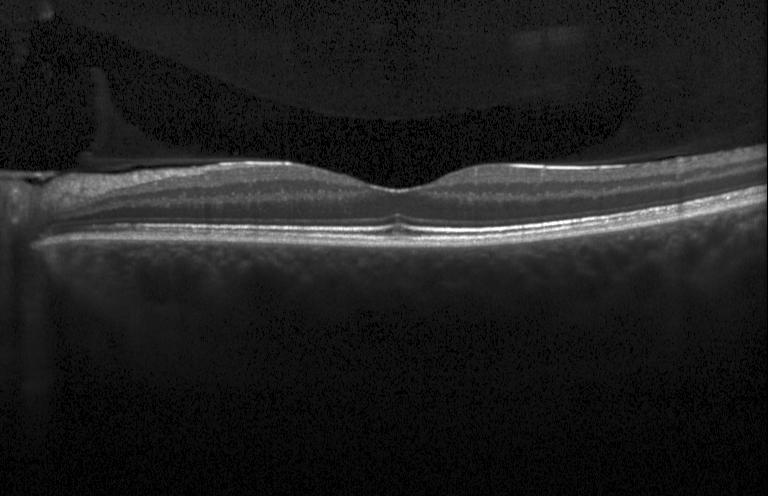

Macular scan. Optical coherence tomography B-scan. Spectral-domain optical coherence tomography.
No choroidal neovascularization, no diabetic macular edema, and no drusen.